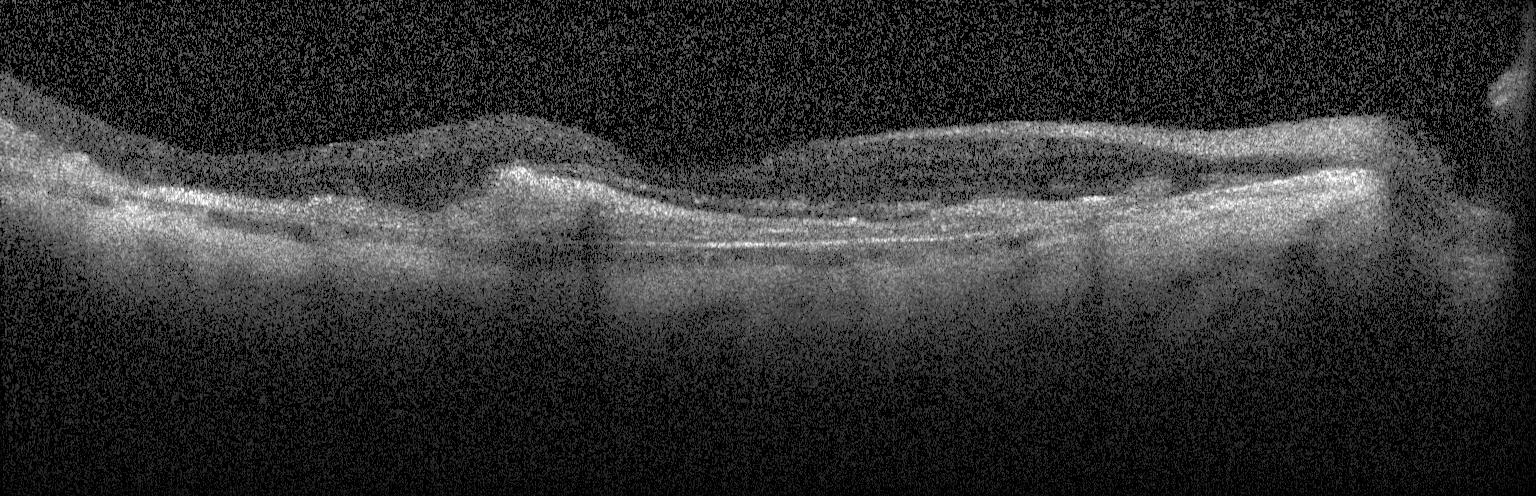
Retinal OCT B-scan — Dx: choroidal neovascularization.